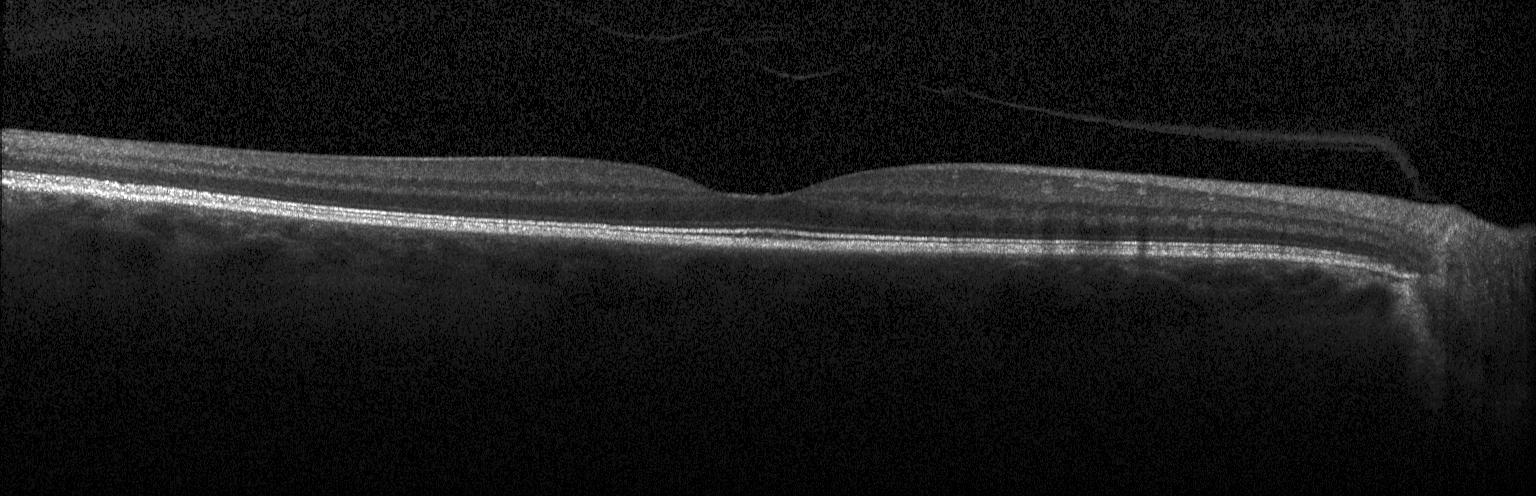
Finding: no choroidal neovascularization, diabetic macular edema, or drusen.